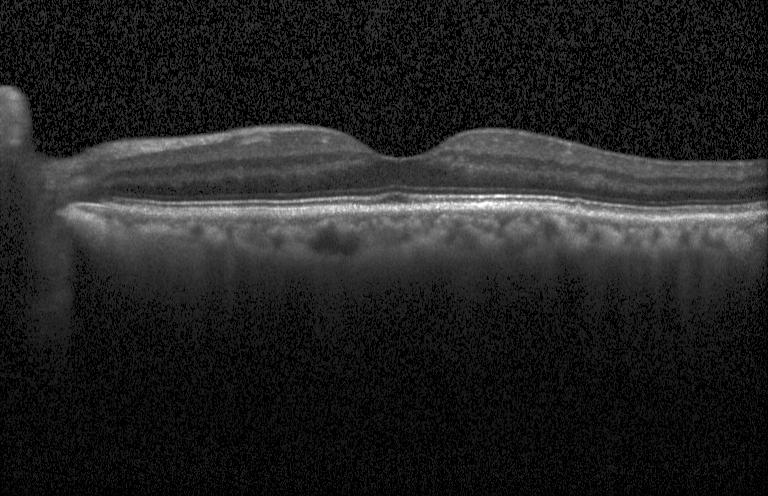
Impression: no CNV, no DME, and no drusen.